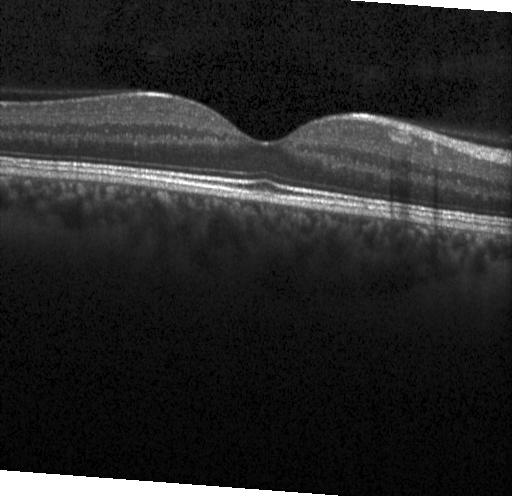

Macular OCT: no CNV, DME, or drusen.